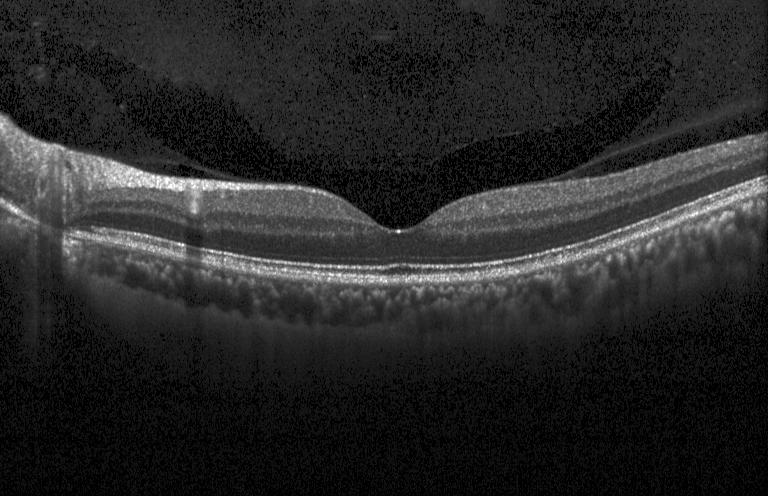

Optical coherence tomography B-scan. Spectral-domain OCT. Horizontal scan through the fovea — Impression: no choroidal neovascularization, diabetic macular edema, or drusen.